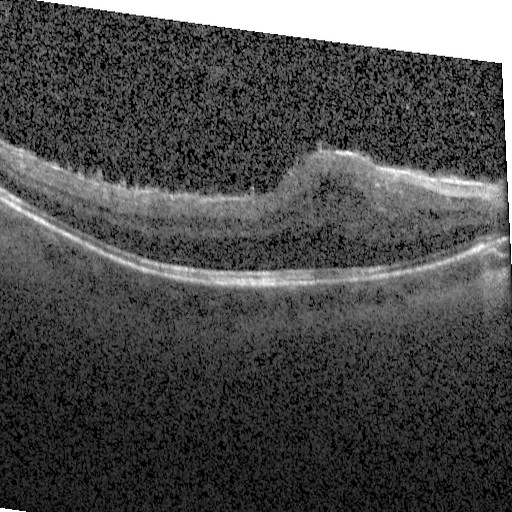

The scan shows diabetic macular edema.